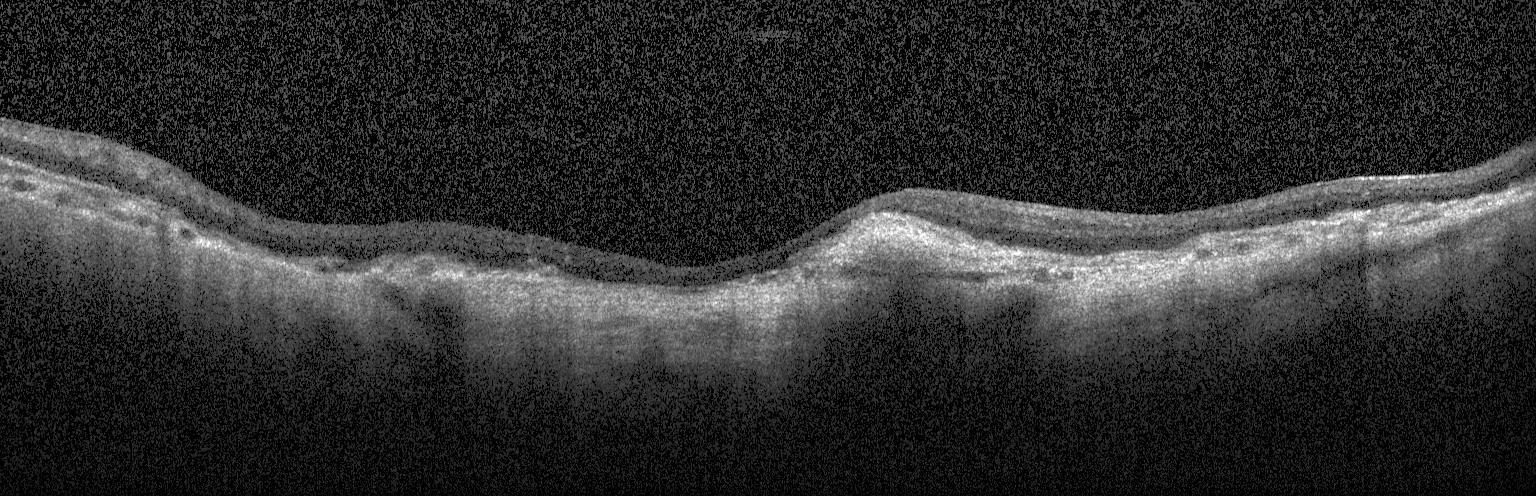

SD-OCT; OCT B-scan; instrument: Heidelberg Spectralis.
Macular OCT: CNV.